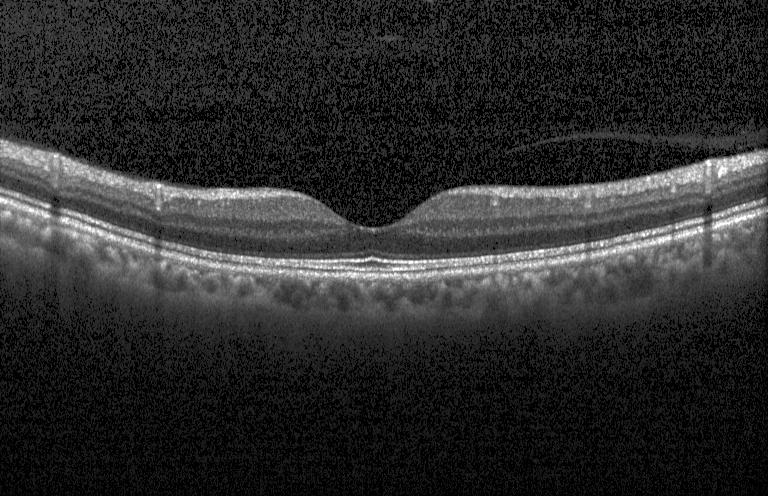
Retinal OCT cross-section
This B-scan demonstrates neither choroidal neovascularization, diabetic macular edema, nor drusen.